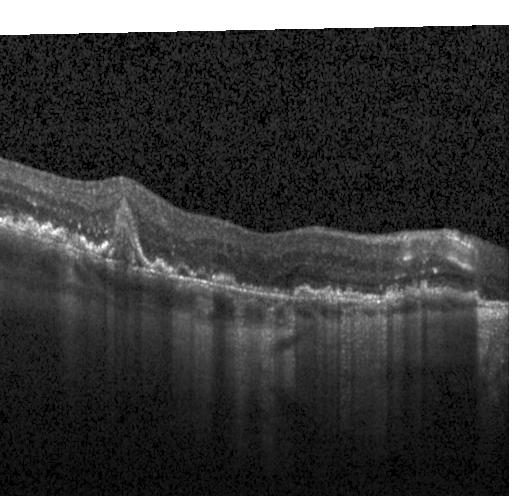 Retinal OCT cross-section.
OCT finding: a choroidal neovascular membrane.